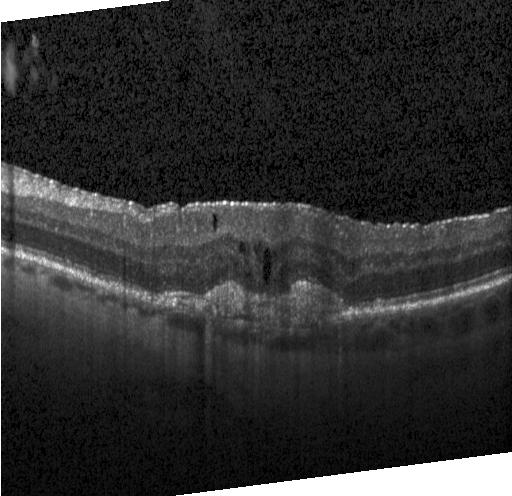

Spectral-domain optical coherence tomography, retinal OCT B-scan, centered on the fovea, Heidelberg Spectralis OCT system
The scan shows a choroidal neovascular membrane.